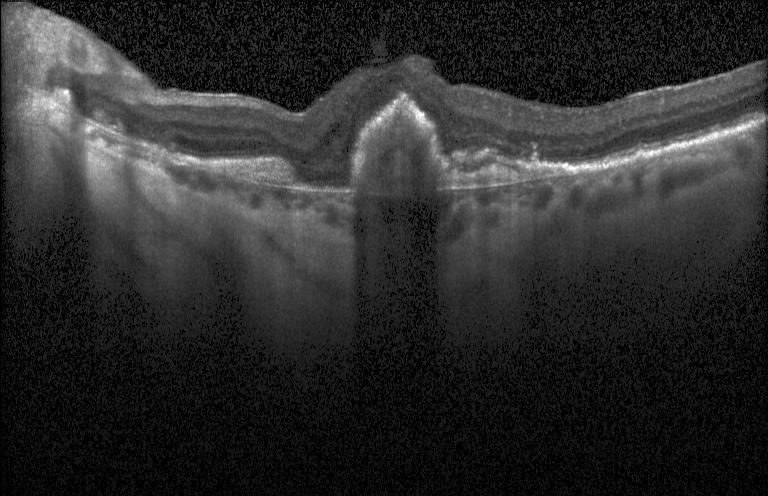

Impression: choroidal neovascularization.